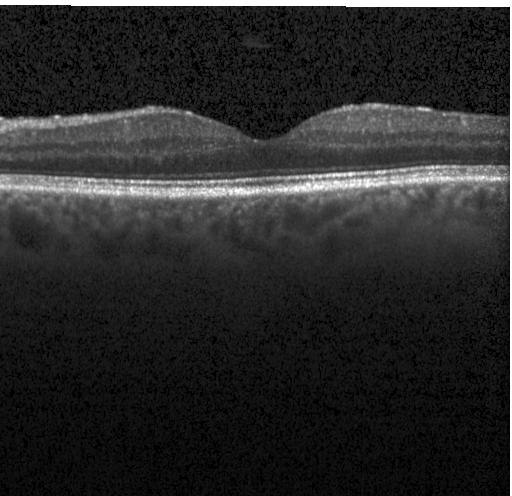

SD-OCT · OCT line scan · through the macula — The scan shows neither choroidal neovascularization, diabetic macular edema, nor drusen.